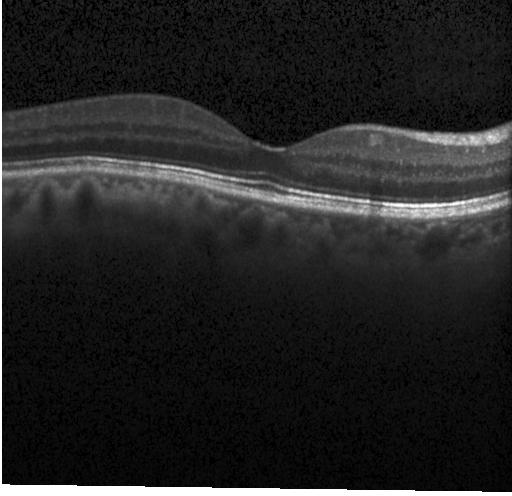 Retinal OCT cross-section
OCT finding: no choroidal neovascularization, diabetic macular edema, or drusen.